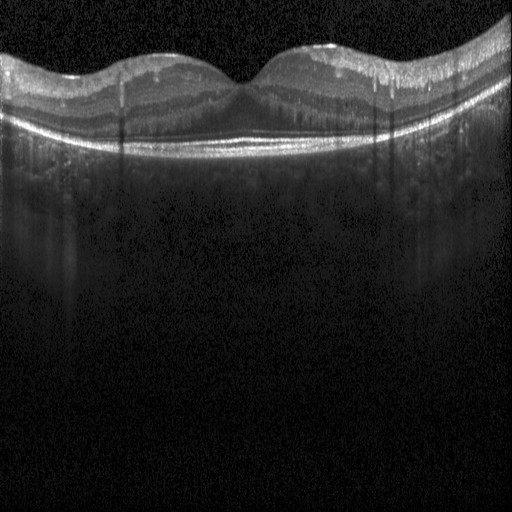 OCT B-scan showing diabetic macular edema.